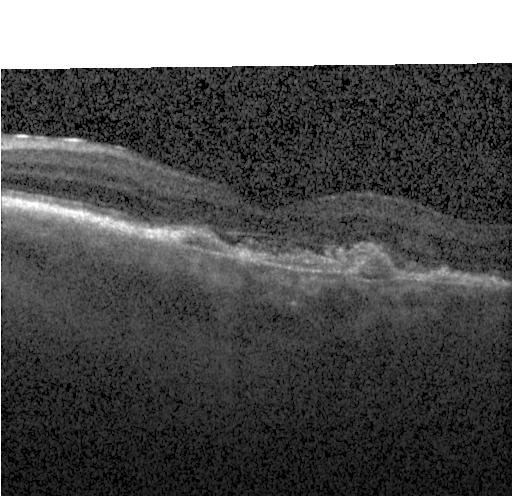 OCT B-scan.
This B-scan demonstrates CNV.